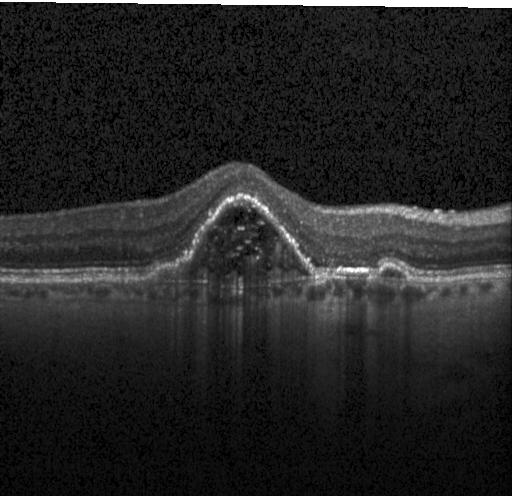 Optical coherence tomography scan
Diagnosis: choroidal neovascularization.